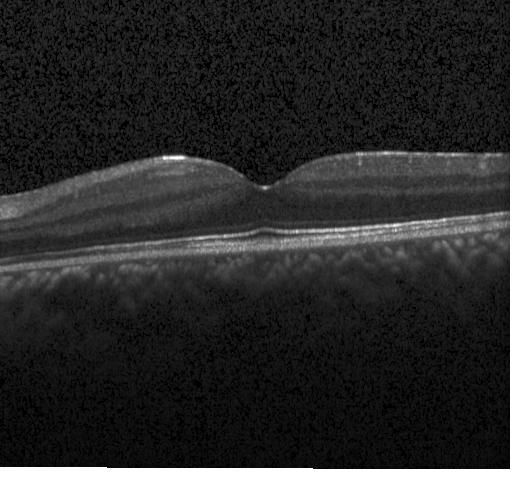

Finding: no choroidal neovascularization, no diabetic macular edema, and no drusen.